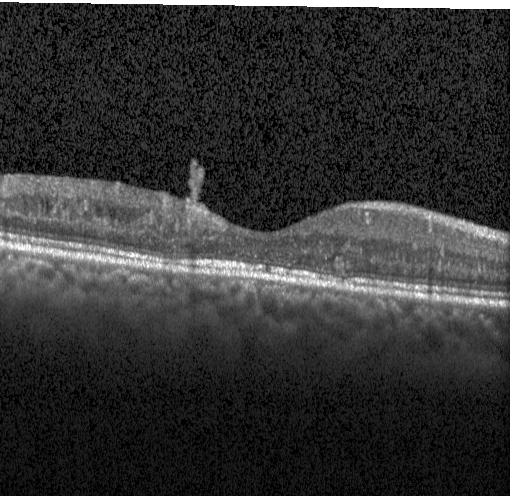
Instrument: Heidelberg Spectralis; SD-OCT; OCT line scan; macular scan.
Impression: diabetic macular edema (DME).